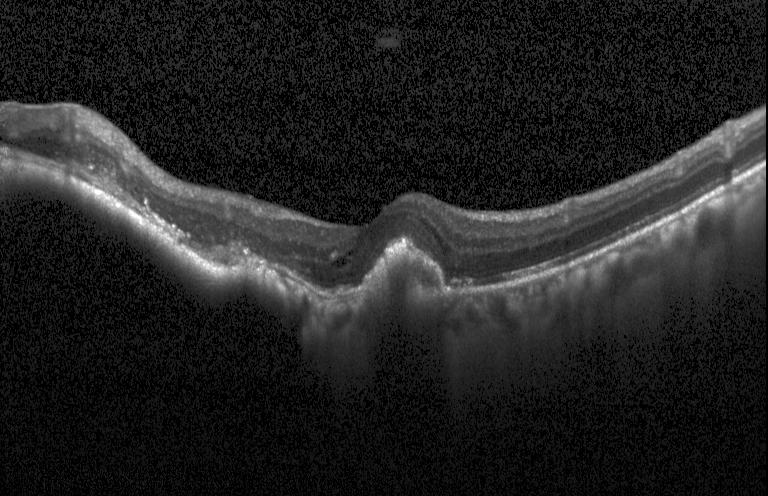
OCT B-scan. Spectral-domain OCT. Instrument: Heidelberg Spectralis. OCT finding: CNV.